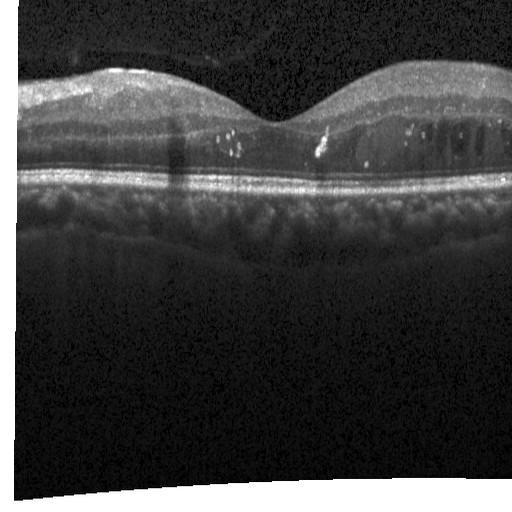

Dx: diabetic macular edema (DME).